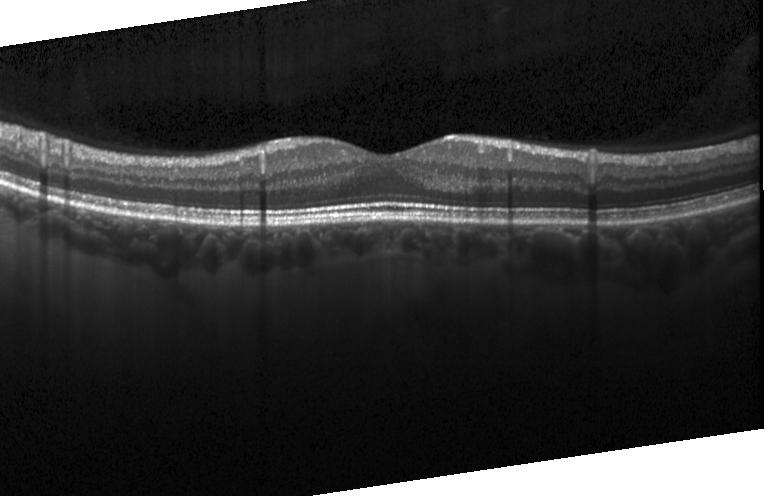 OCT B-scan; instrument: Heidelberg Spectralis — This B-scan demonstrates neither choroidal neovascularization, diabetic macular edema, nor drusen.